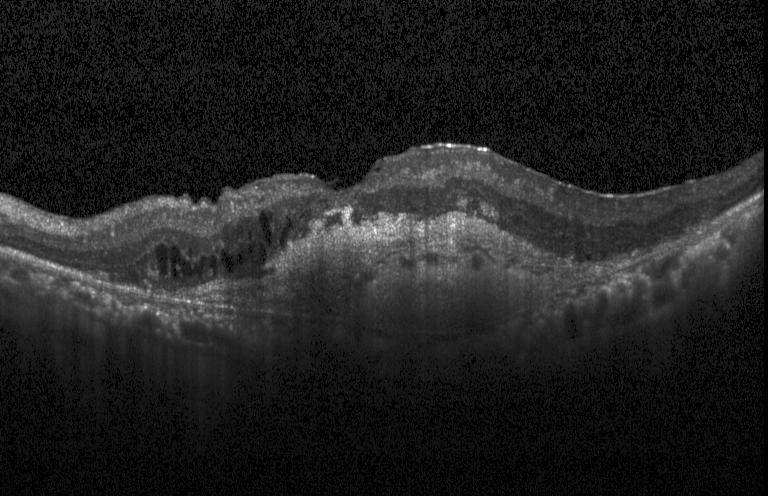 Centered on the fovea; retinal OCT cross-section
Impression: choroidal neovascularization.